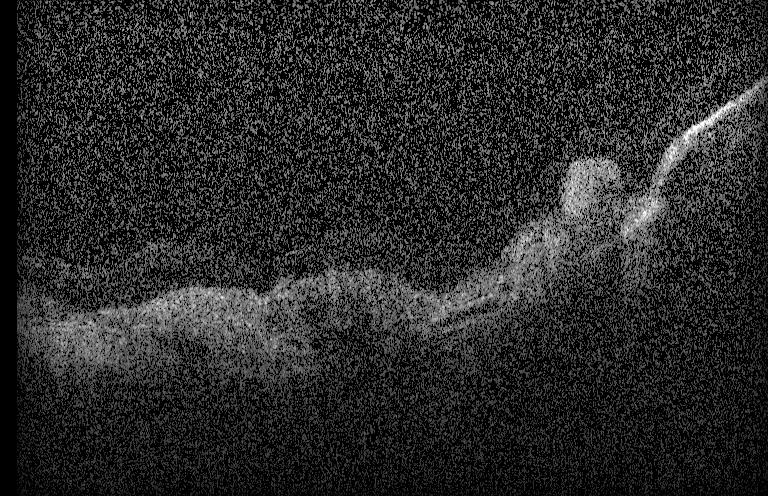
Centered on the fovea. Spectral-domain OCT. Heidelberg Spectralis OCT system. OCT line scan. Impression: a choroidal neovascular membrane.